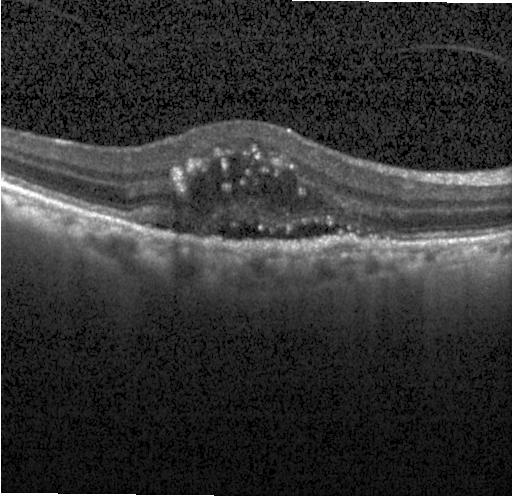

Macular OCT: choroidal neovascularization (CNV).